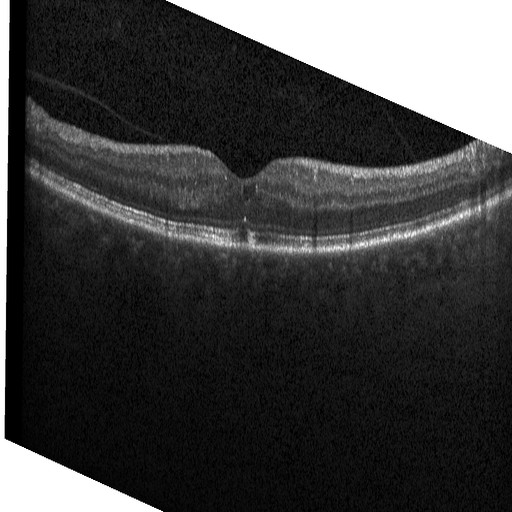 Spectral-domain optical coherence tomography · retinal OCT cross-section — Impression: diabetic macular edema (DME).